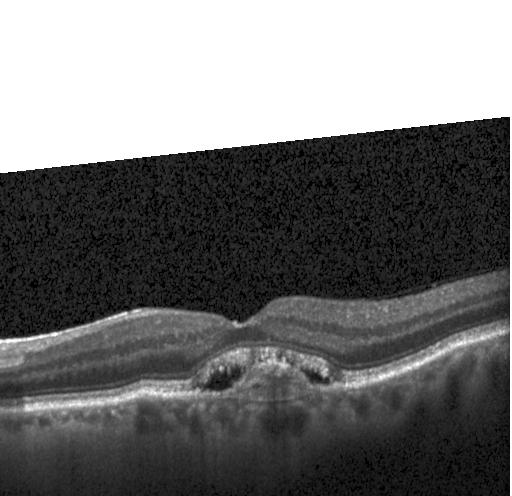 OCT finding: a choroidal neovascular membrane.